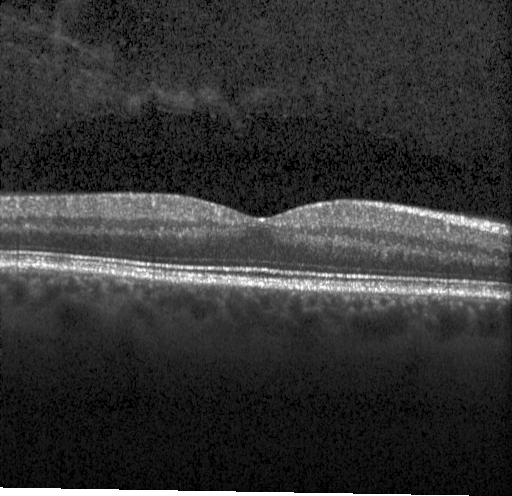
Heidelberg Spectralis. Spectral-domain OCT. Optical coherence tomography scan. Through the macula.
Neither choroidal neovascularization, diabetic macular edema, nor drusen.